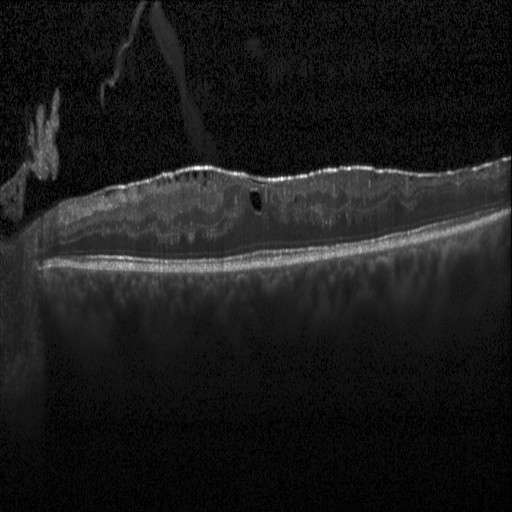
Heidelberg Spectralis · optical coherence tomography B-scan — The scan shows DME.